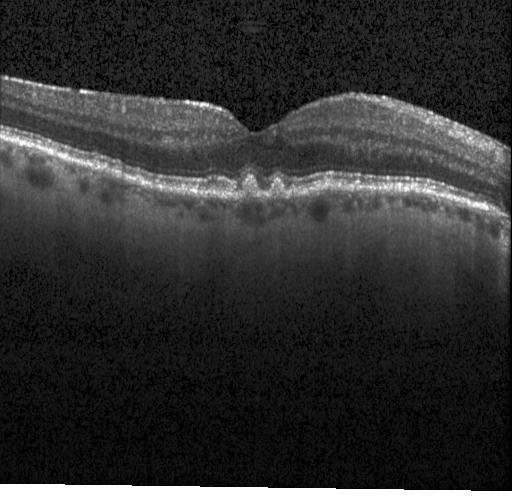

Multiple drusen.